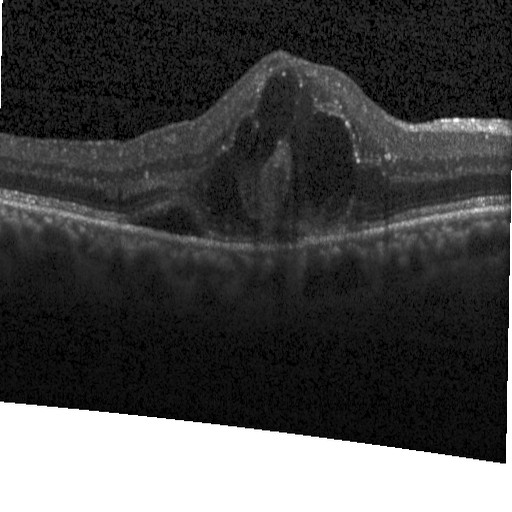
OCT B-scan · through the macula.
Impression: diabetic macular edema.